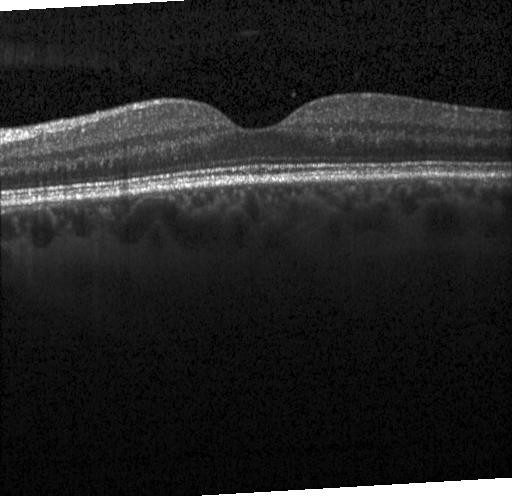

Centered on the fovea · OCT B-scan · instrument: Heidelberg Spectralis. Macular OCT: neither choroidal neovascularization, diabetic macular edema, nor drusen.